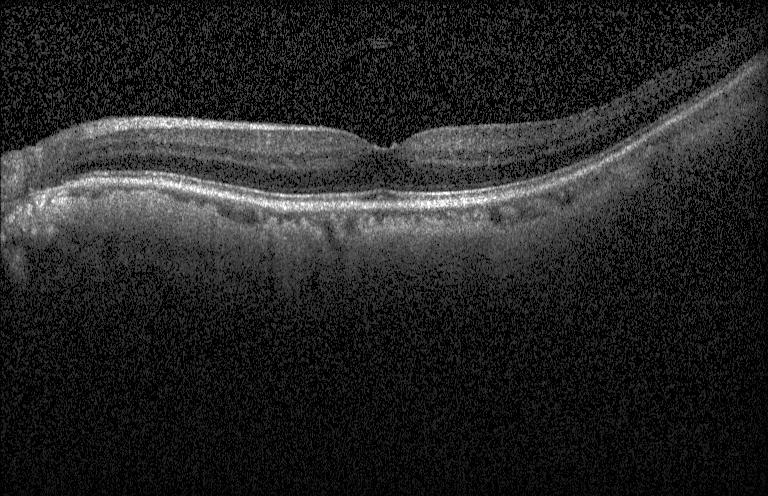

Finding: no CNV, no DME, and no drusen.